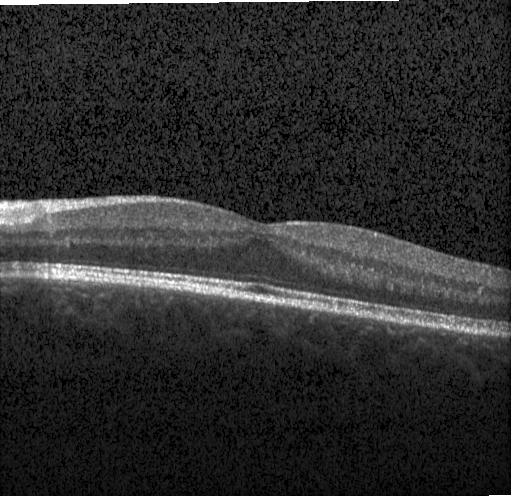

Optical coherence tomography B-scan.
Diagnosis: no CNV, DME, or drusen.